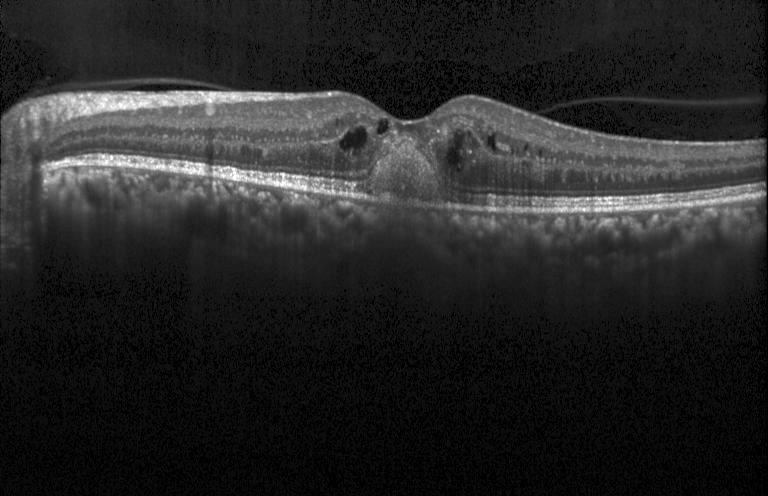

Dx: choroidal neovascularization (CNV).